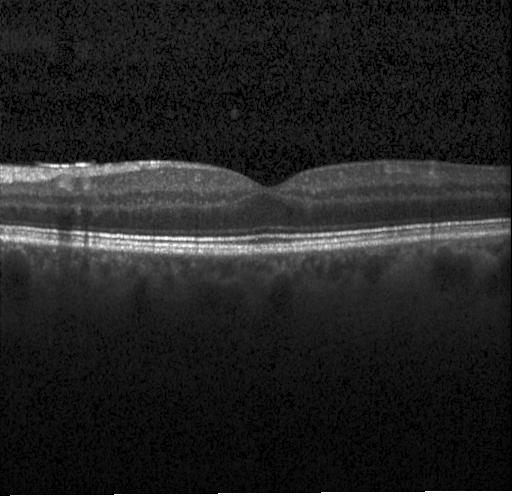 Heidelberg Spectralis OCT system · retinal OCT B-scan · spectral-domain optical coherence tomography · macular scan.
Neither CNV, DME, nor drusen.